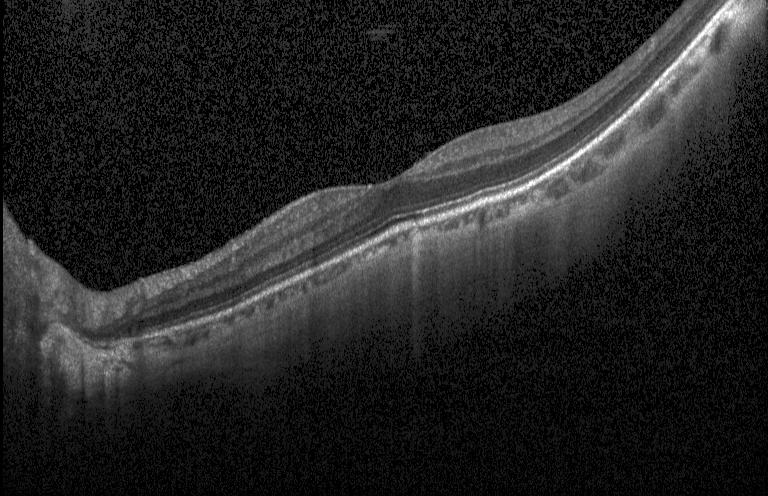

Optical coherence tomography B-scan — Diagnosis: no evidence of choroidal neovascularization, diabetic macular edema, or drusen.